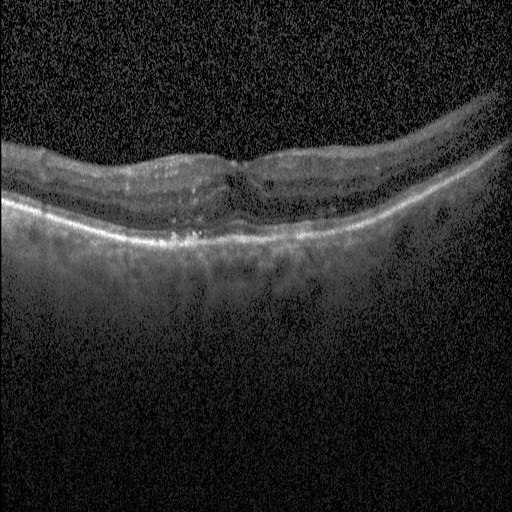
Retinal OCT B-scan — The scan shows DME.